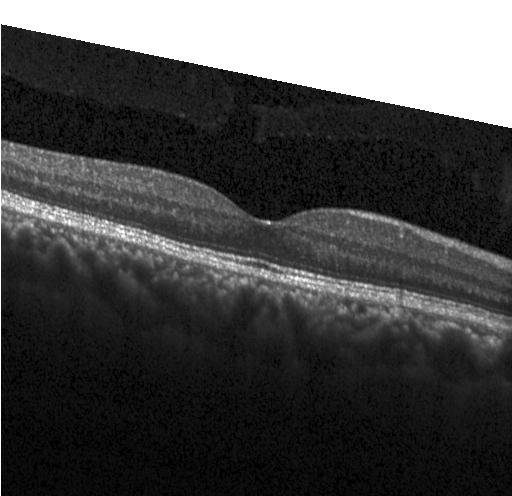
The scan shows no choroidal neovascularization, no diabetic macular edema, and no drusen.